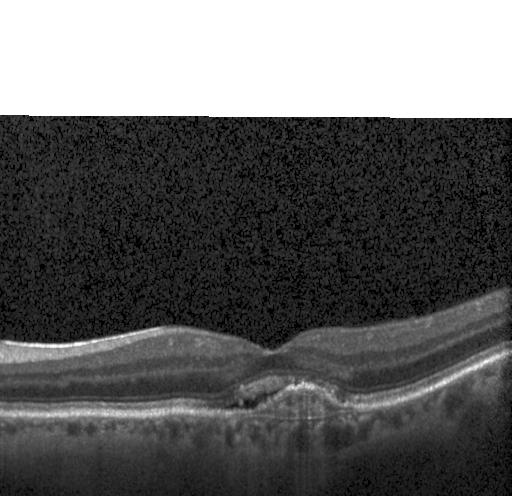
Diagnosis: choroidal neovascularization (CNV).